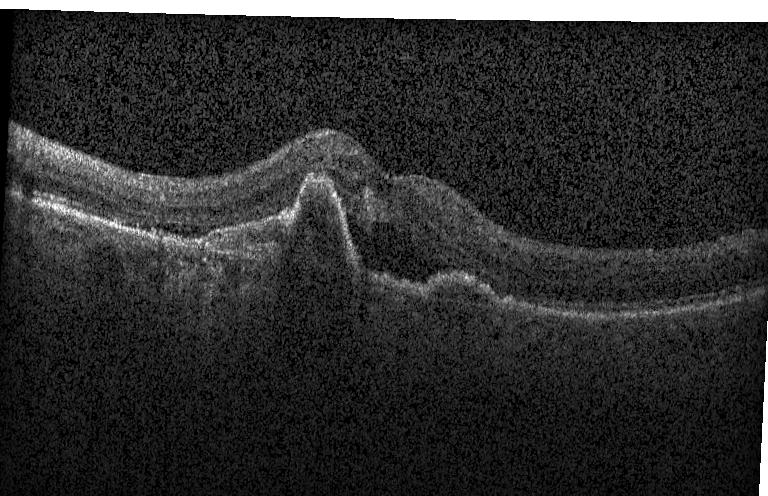
Impression: a choroidal neovascular membrane.